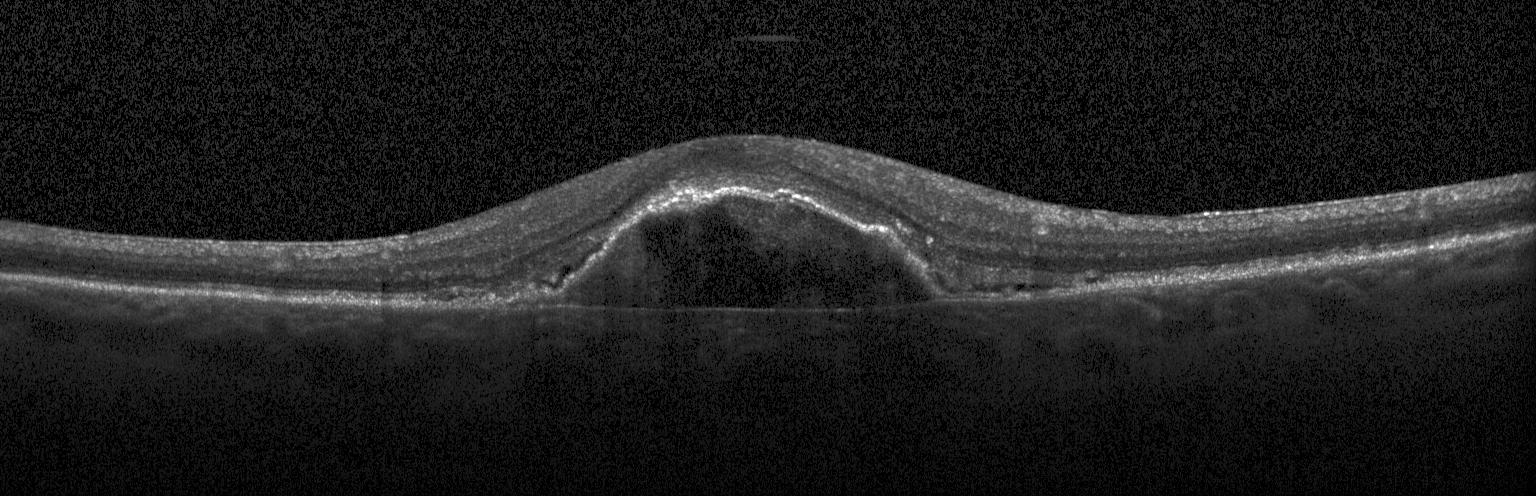
Diagnosis: CNV.